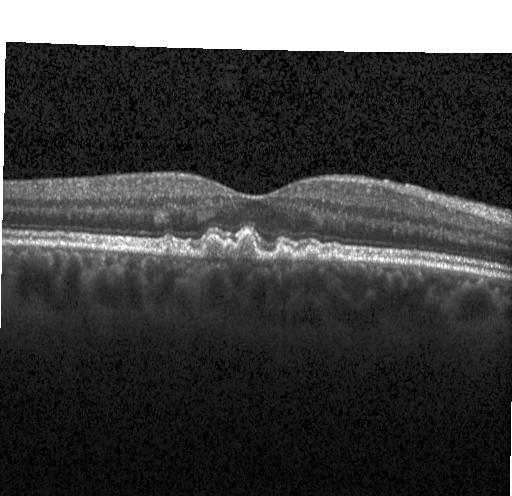 Retinal OCT B-scan, Heidelberg Spectralis OCT system.
Assessment: drusen.